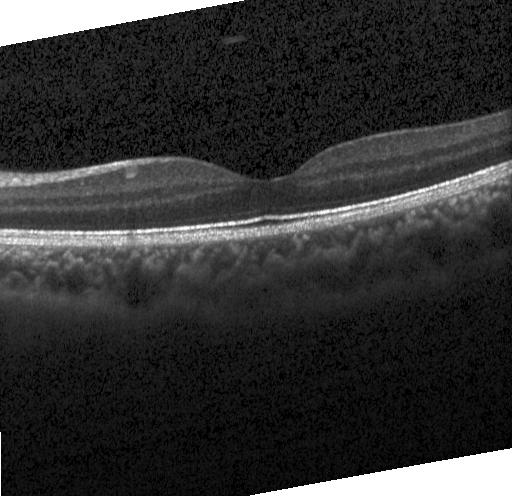
This B-scan demonstrates no choroidal neovascularization, diabetic macular edema, or drusen.